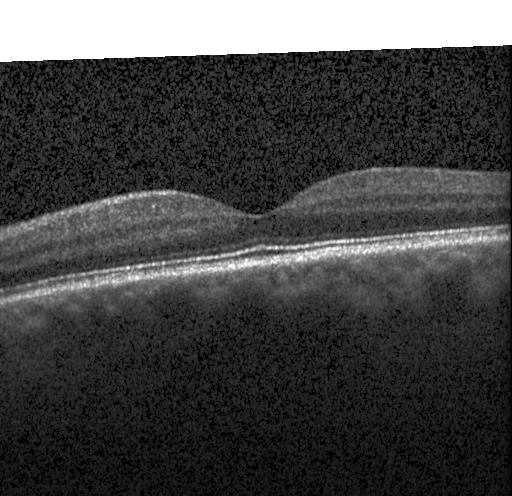

Optical coherence tomography B-scan — This B-scan demonstrates no choroidal neovascularization, no diabetic macular edema, and no drusen.